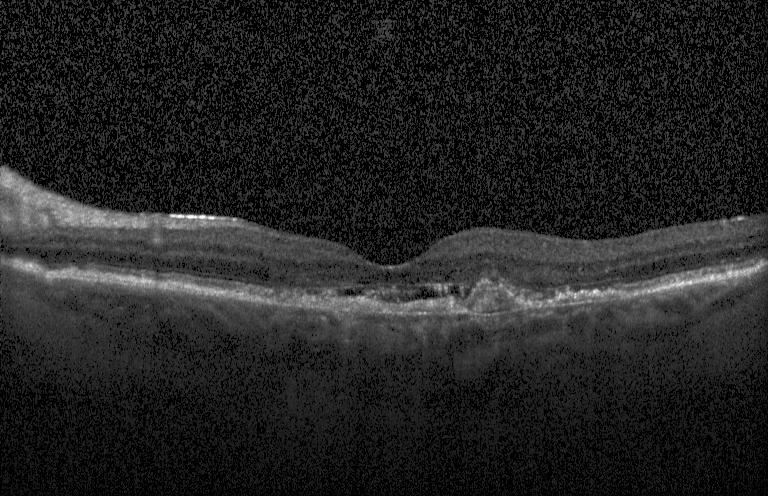 Retinal OCT cross-section. Acquired on a Heidelberg Spectralis.
Diagnosis: a choroidal neovascular membrane.